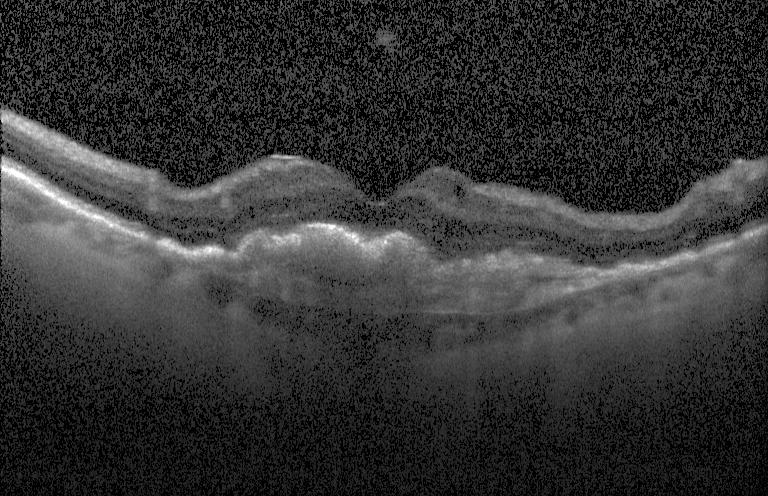 OCT line scan. Finding: a choroidal neovascular membrane.